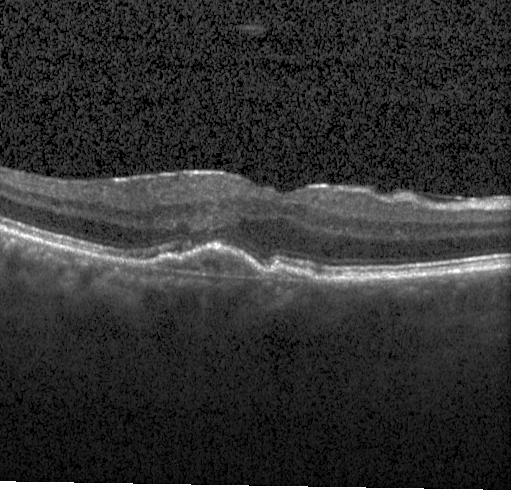
OCT line scan. Finding: a choroidal neovascular membrane.